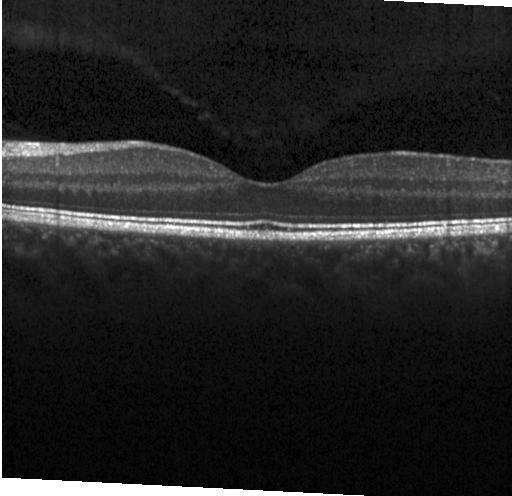 This B-scan demonstrates neither choroidal neovascularization, diabetic macular edema, nor drusen.